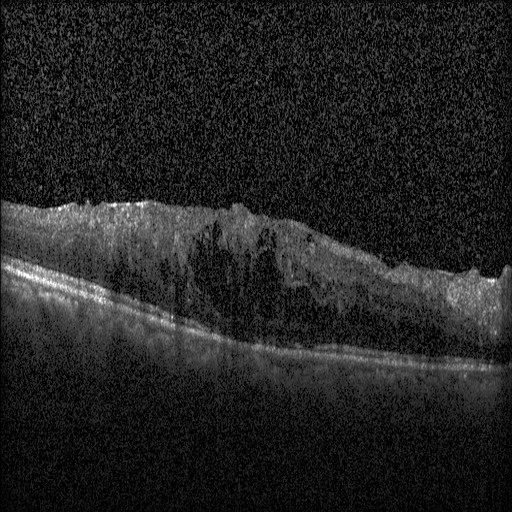 Optical coherence tomography scan · spectral-domain OCT · centered on the fovea · acquired on a Heidelberg Spectralis.
Diabetic macular edema.